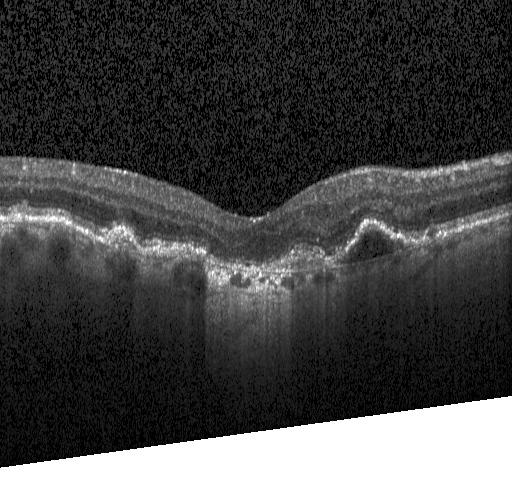 Impression: a choroidal neovascular membrane.